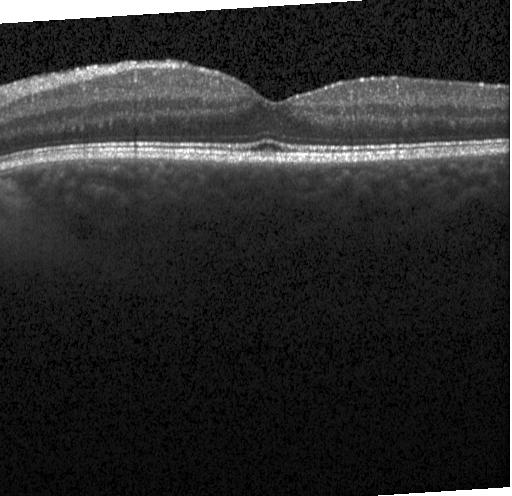
Finding: neither choroidal neovascularization, diabetic macular edema, nor drusen.